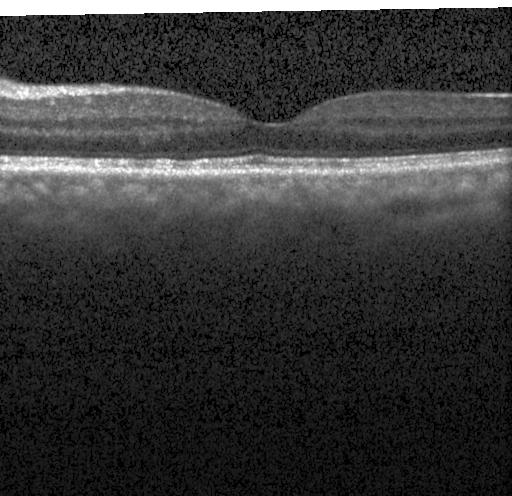
SD-OCT, macular scan, Heidelberg Spectralis OCT system, retinal OCT cross-section — No choroidal neovascularization, no diabetic macular edema, and no drusen.